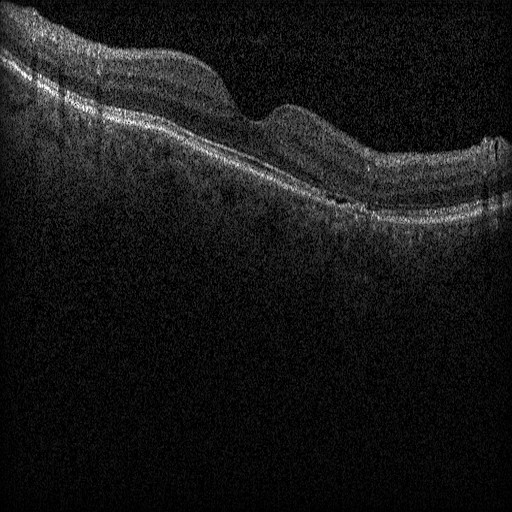

Acquired on a Heidelberg Spectralis. Spectral-domain optical coherence tomography. Retinal OCT cross-section. Centered on the fovea
Diagnosis: DME.